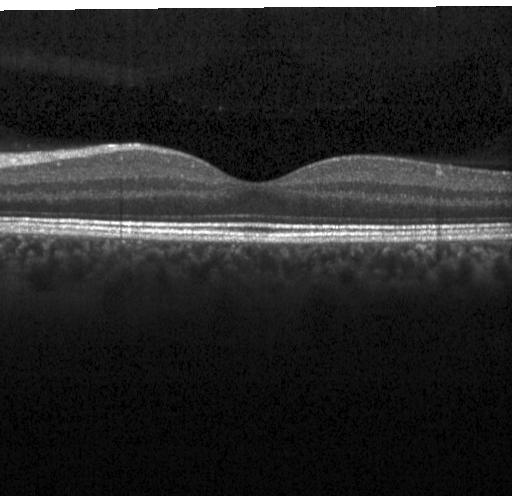

Impression: no choroidal neovascularization, diabetic macular edema, or drusen.